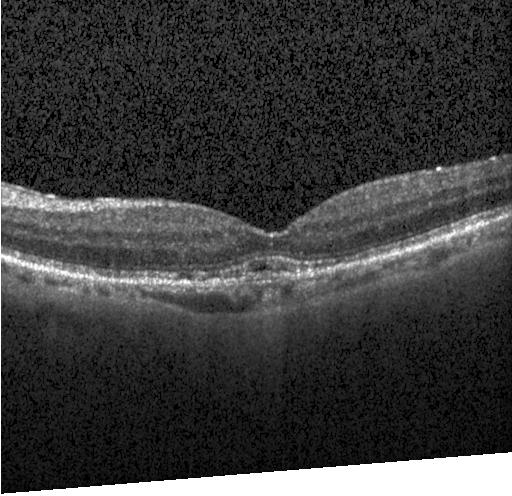

OCT line scan · Heidelberg Spectralis OCT system. Finding: a choroidal neovascular membrane.